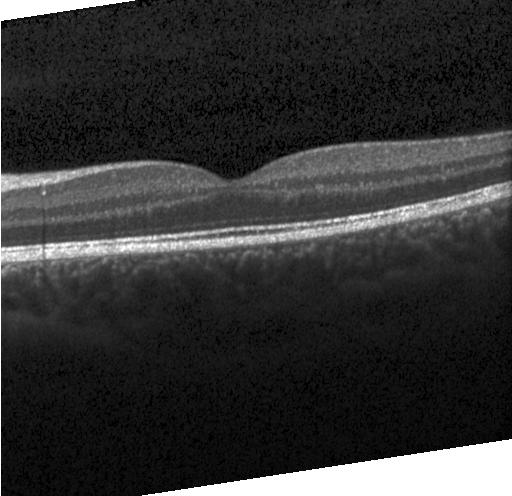
Retinal OCT cross-section; spectral-domain OCT.
Macular OCT: neither choroidal neovascularization, diabetic macular edema, nor drusen.